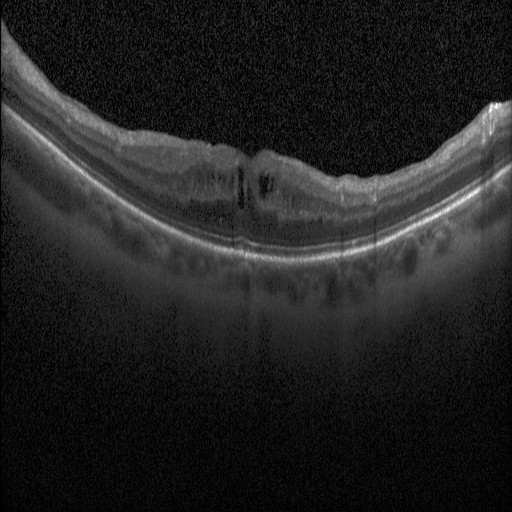 Diagnosis: diabetic macular edema (DME).